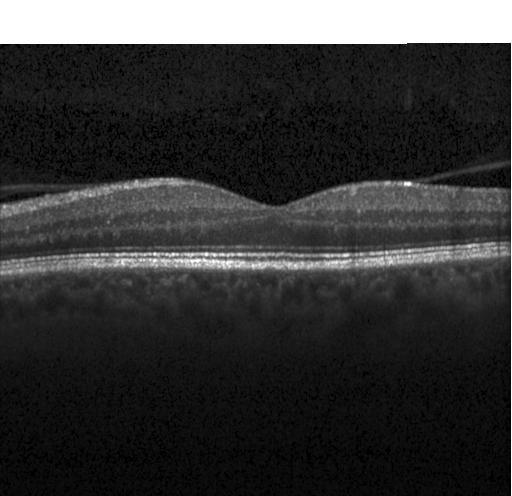

Retinal OCT cross-section showing no choroidal neovascularization, no diabetic macular edema, and no drusen.